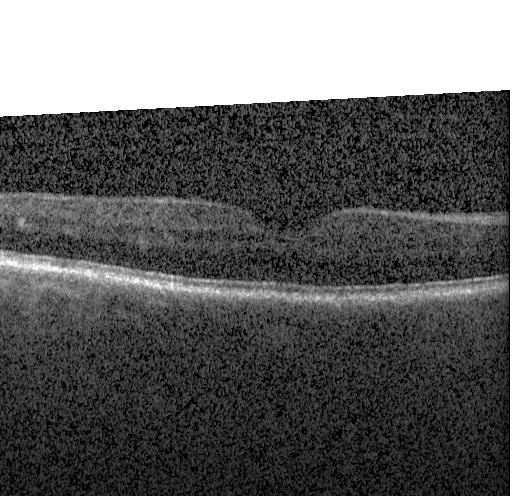

Finding: no choroidal neovascularization, diabetic macular edema, or drusen.